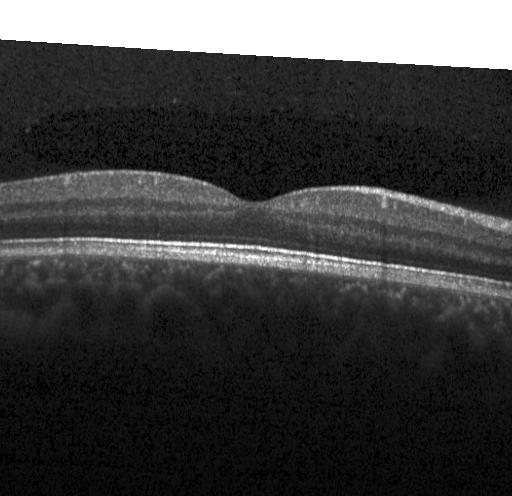

Retinal OCT cross-section · fovea-centered
This B-scan demonstrates no choroidal neovascularization, no diabetic macular edema, and no drusen.